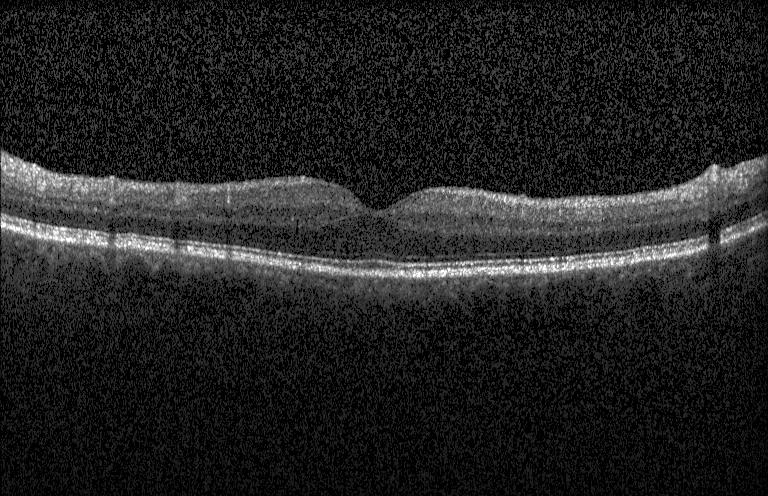 Retinal OCT cross-section. Finding: neither choroidal neovascularization, diabetic macular edema, nor drusen.